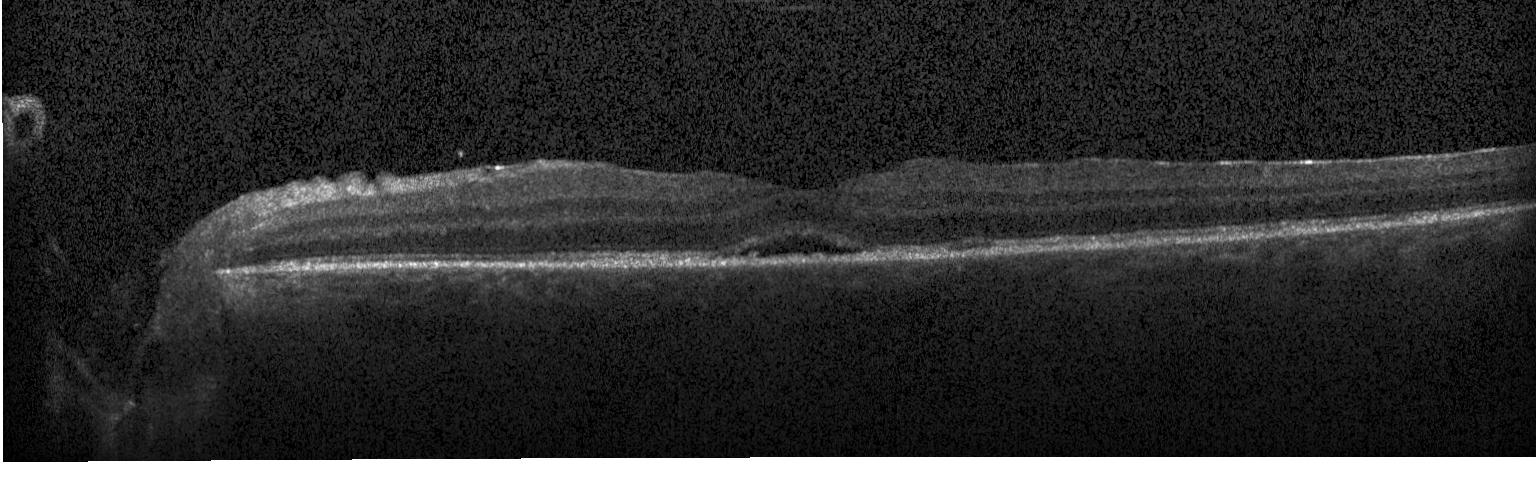
OCT scan showing a choroidal neovascular membrane.